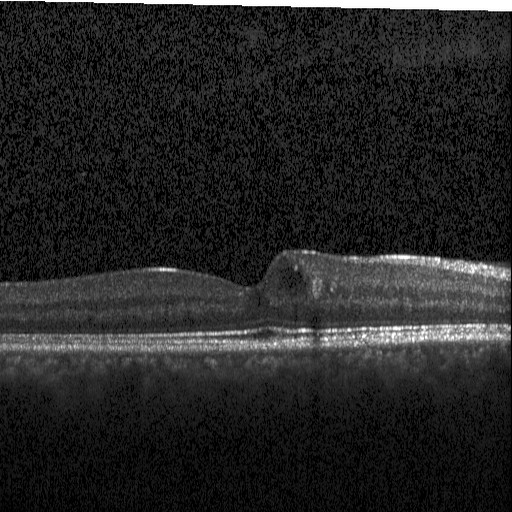
Spectral-domain OCT B-scan: diabetic macular edema (DME).